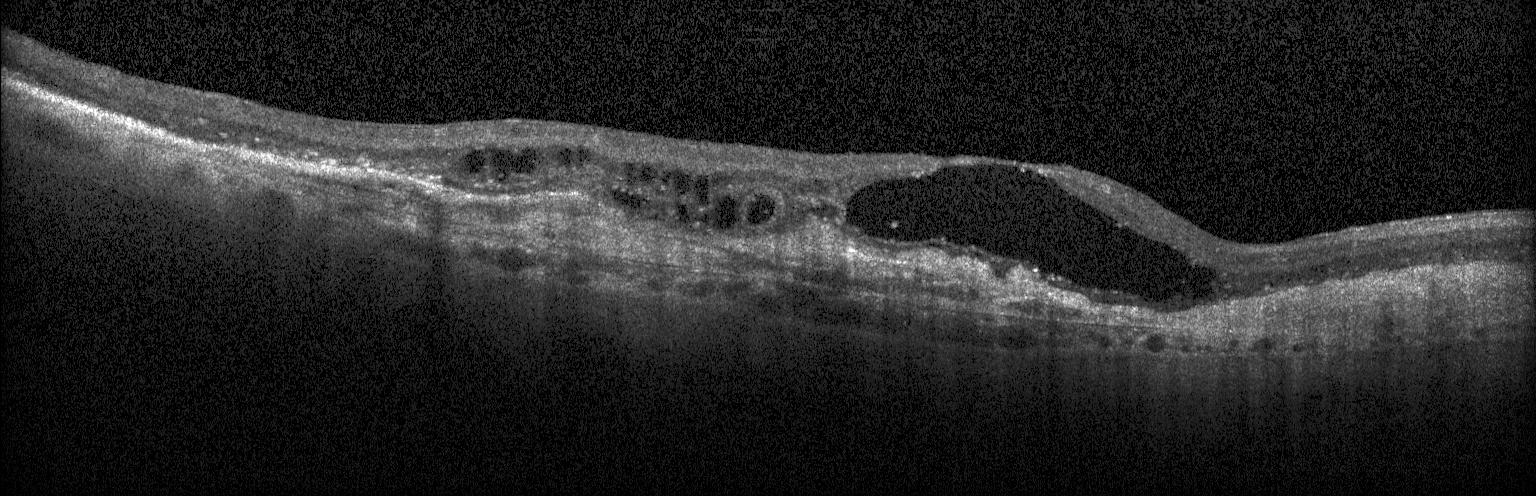

Optical coherence tomography B-scan · acquired on a Heidelberg Spectralis · SD-OCT · centered on the fovea.
Diagnosis: a choroidal neovascular membrane.